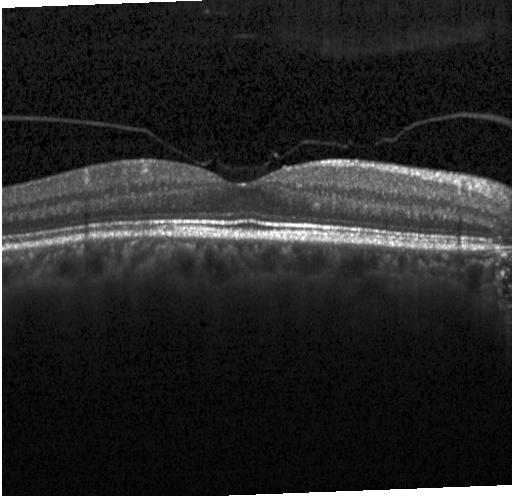 OCT finding: no CNV, DME, or drusen.